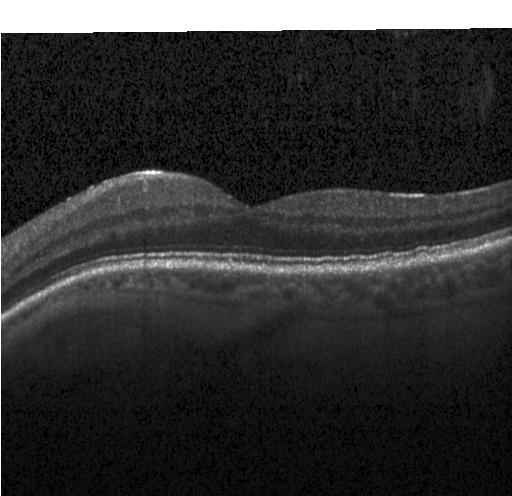
Macular scan; retinal OCT B-scan
Finding: multiple drusen.